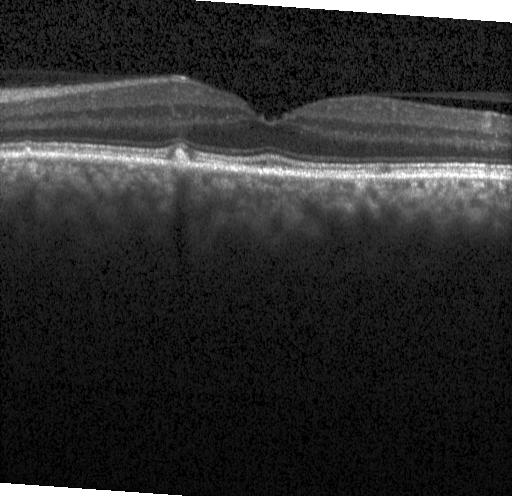 Dx: multiple drusen.